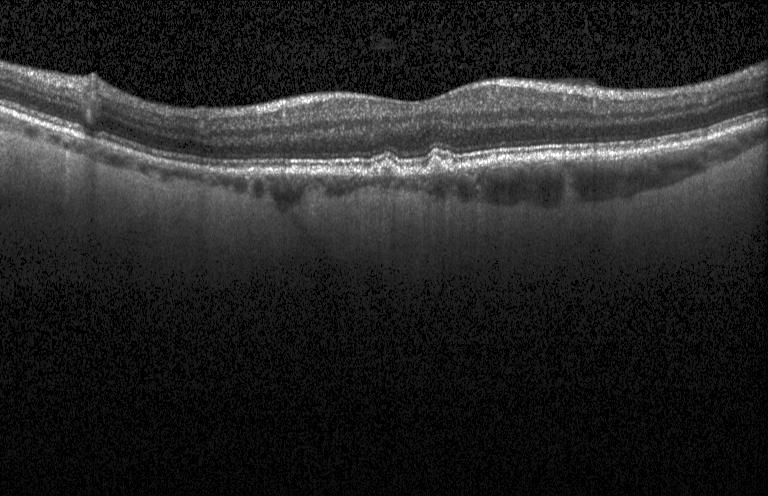
Through the macula, SD-OCT, retinal OCT cross-section. Impression: multiple drusen.